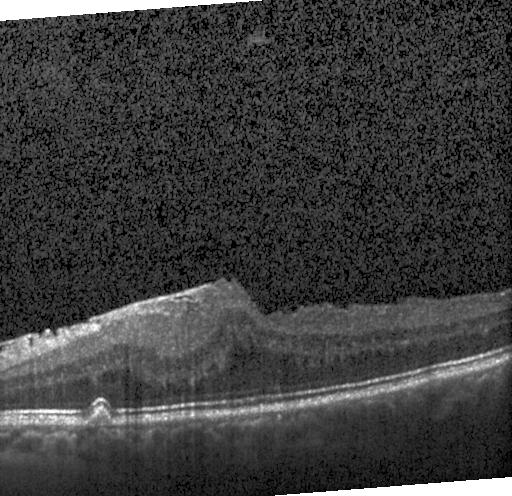 Macular scan. Spectral-domain OCT. Retinal OCT B-scan. Instrument: Heidelberg Spectralis. Impression: multiple drusen.